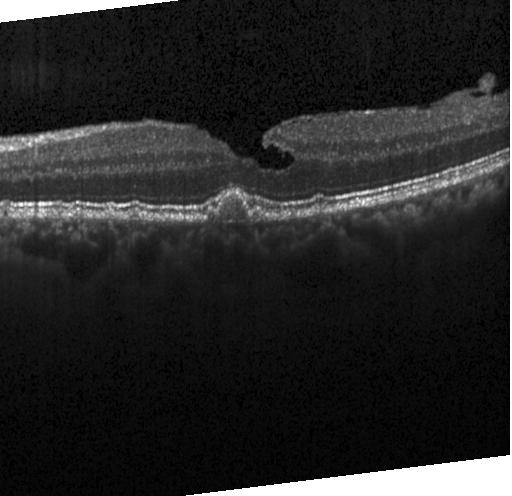

Dx: sub-RPE drusenoid deposits.